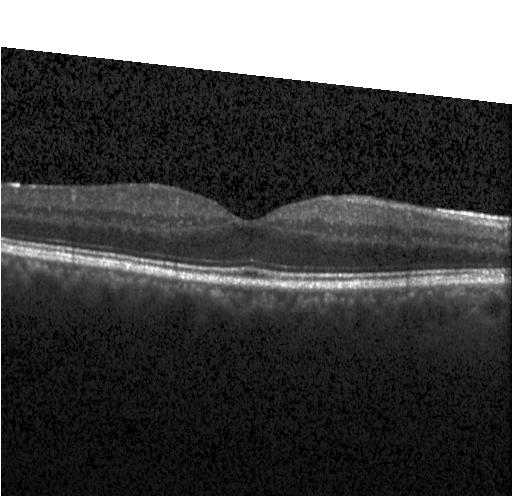
OCT scan showing no choroidal neovascularization, diabetic macular edema, or drusen.